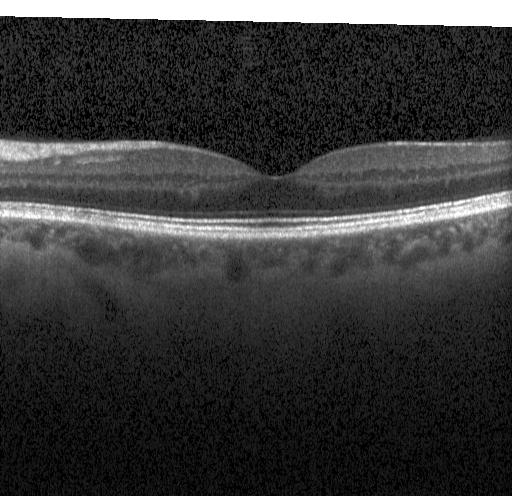
Assessment: no CNV, DME, or drusen.